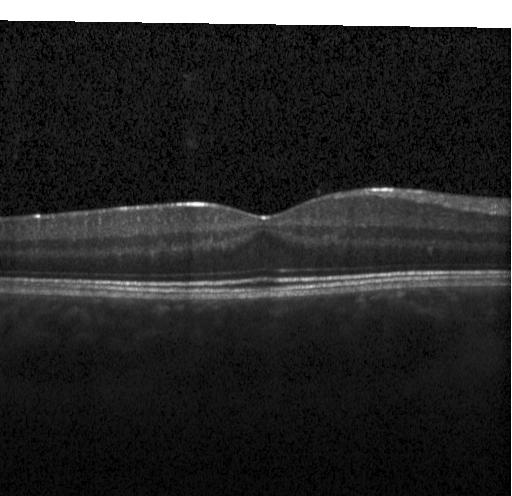 Through the macula, instrument: Heidelberg Spectralis, optical coherence tomography B-scan, SD-OCT
Impression: neither choroidal neovascularization, diabetic macular edema, nor drusen.